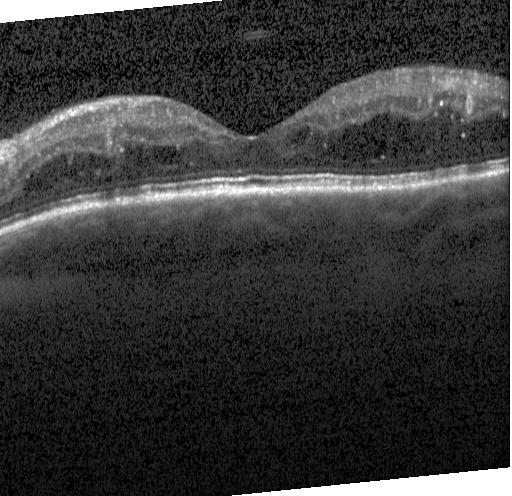 Macular scan · OCT B-scan.
Finding: diabetic macular edema (DME).